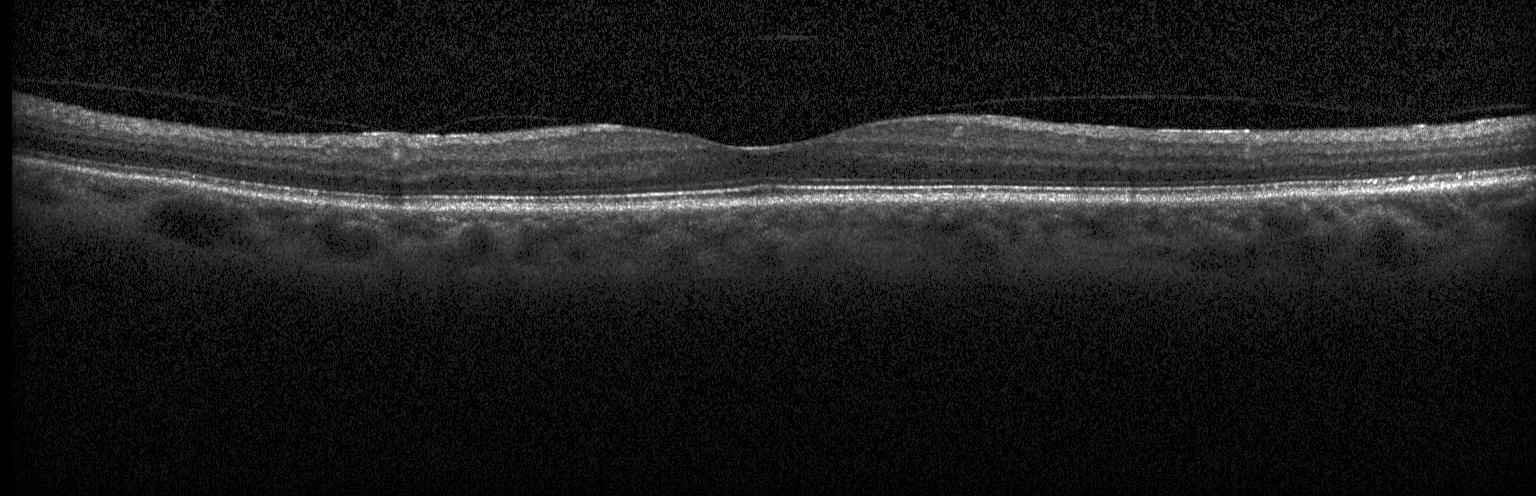 Spectral-domain OCT; fovea-centered; OCT B-scan — The scan shows no evidence of CNV, DME, or drusen.